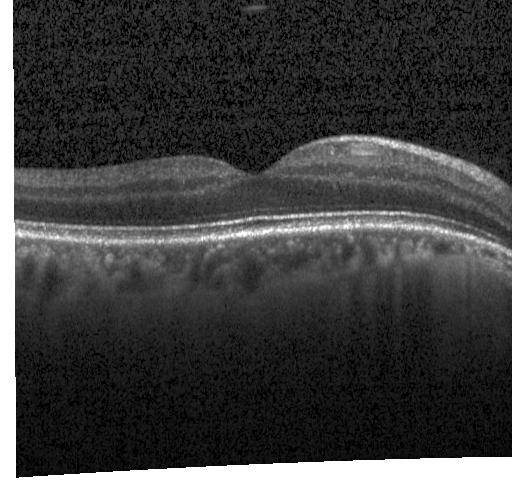
OCT line scan. Diagnosis: neither CNV, DME, nor drusen.